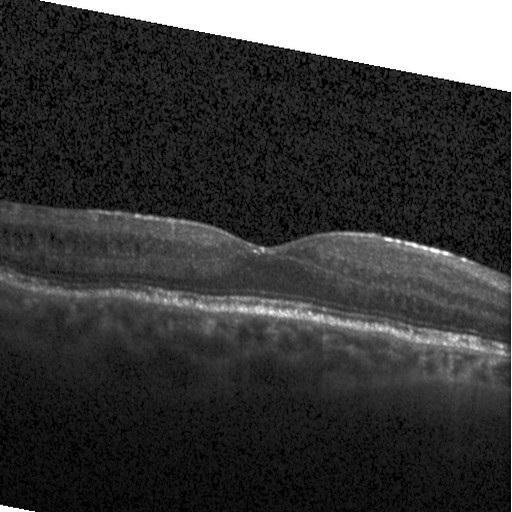
Spectral-domain optical coherence tomography, macular scan, retinal OCT B-scan, Heidelberg Spectralis. The scan shows diabetic macular edema (DME).